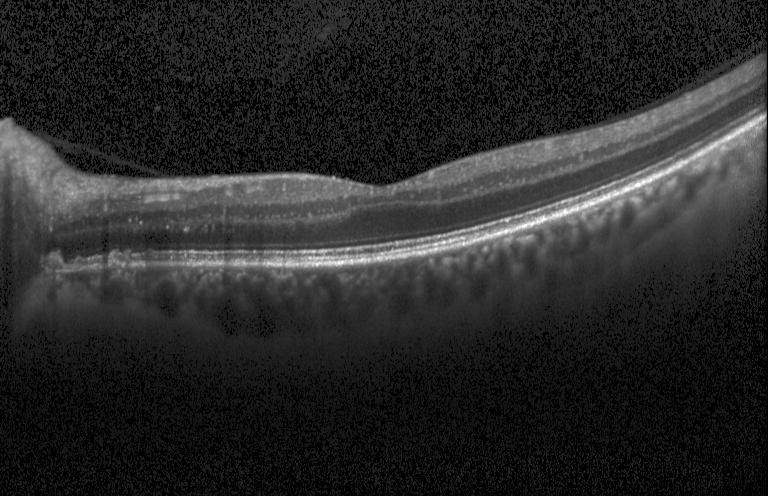
Dx: multiple drusen.